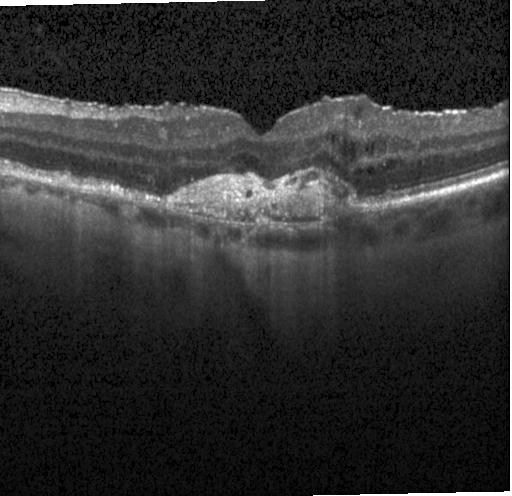 OCT scan showing a choroidal neovascular membrane.